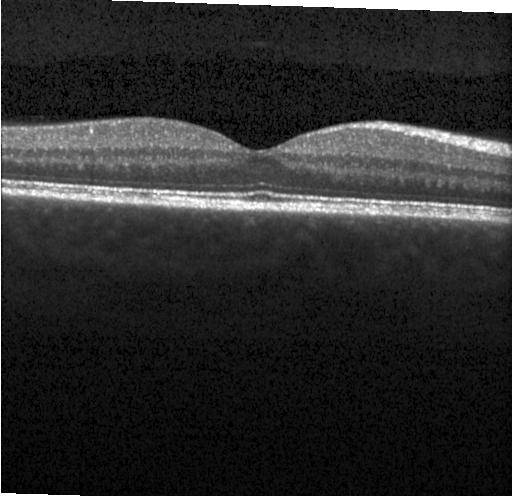 Through the macula; spectral-domain optical coherence tomography; optical coherence tomography scan. Impression: neither choroidal neovascularization, diabetic macular edema, nor drusen.